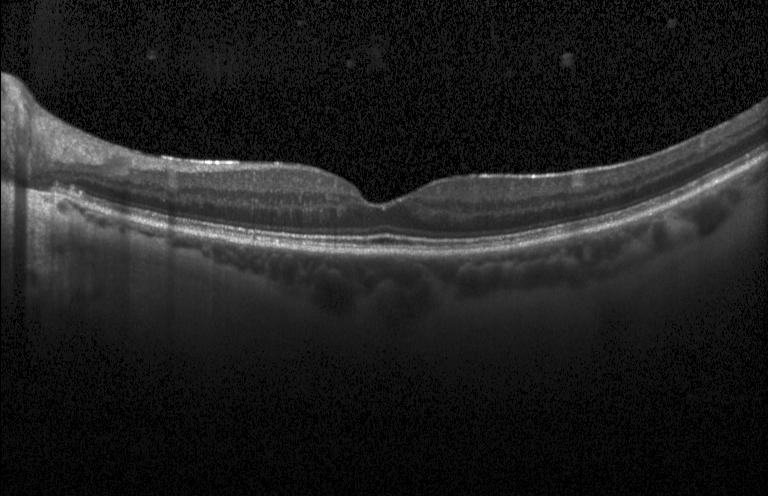 Heidelberg Spectralis OCT system; centered on the fovea; optical coherence tomography scan.
No evidence of choroidal neovascularization, diabetic macular edema, or drusen.